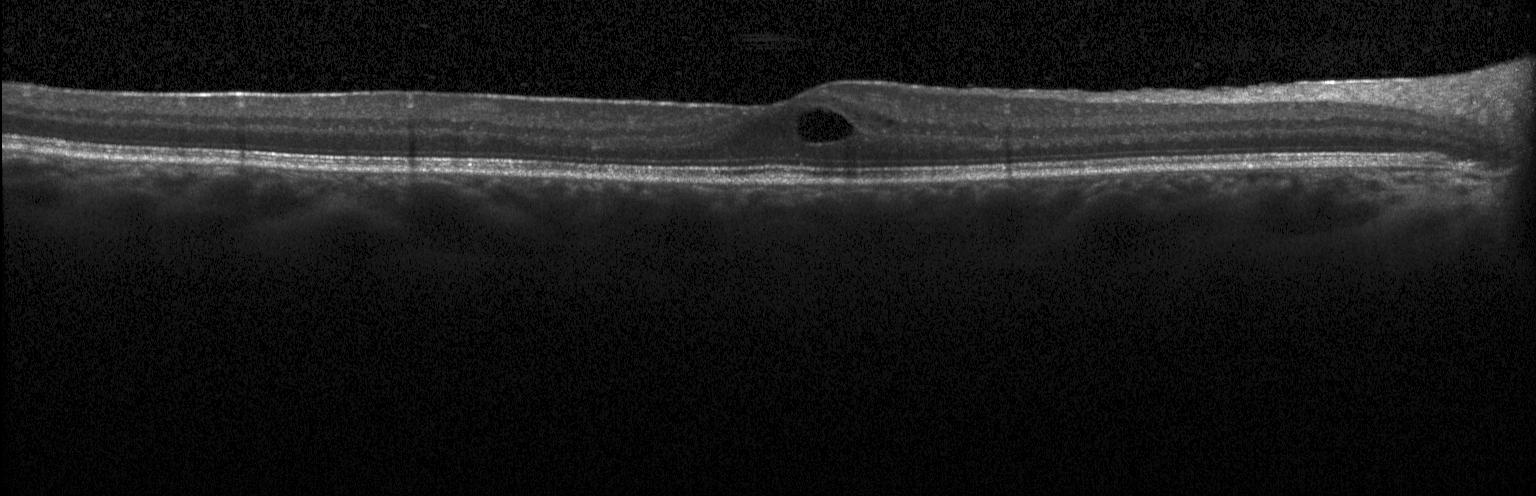
Diagnosis: DME.